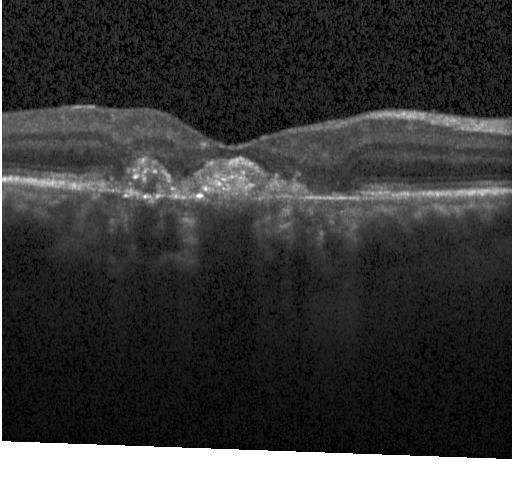 Macular OCT demonstrating a choroidal neovascular membrane.